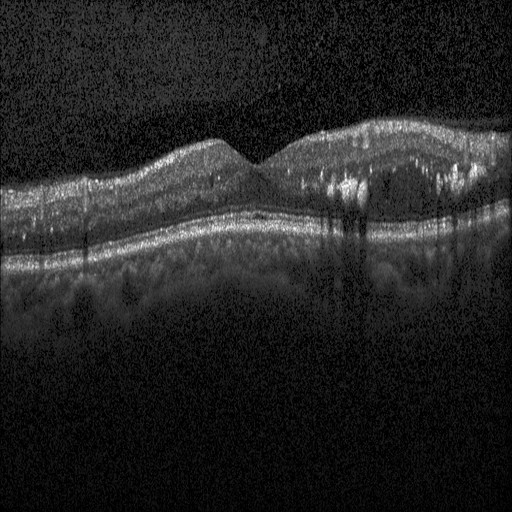
Macular OCT demonstrating diabetic macular edema.